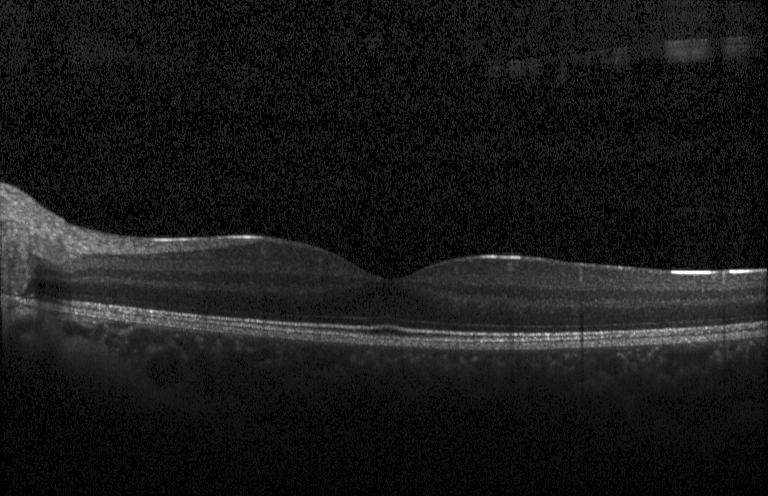
Retinal OCT cross-section showing no evidence of choroidal neovascularization, diabetic macular edema, or drusen.